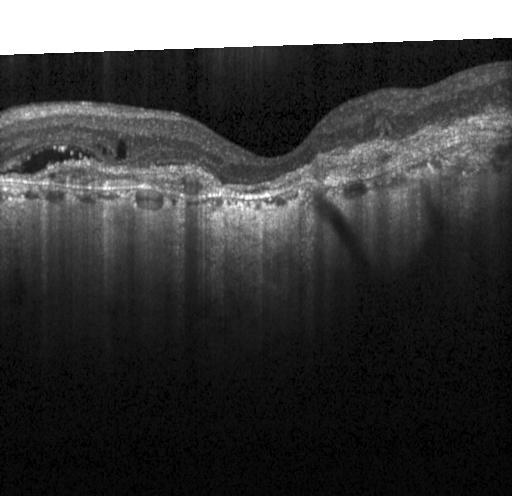 Optical coherence tomography B-scan · horizontal scan through the fovea · spectral-domain optical coherence tomography · Heidelberg Spectralis OCT system. Assessment: choroidal neovascularization (CNV).